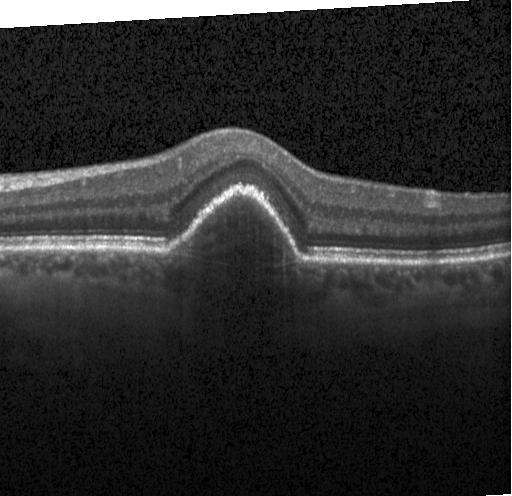

Optical coherence tomography scan — Assessment: a choroidal neovascular membrane.